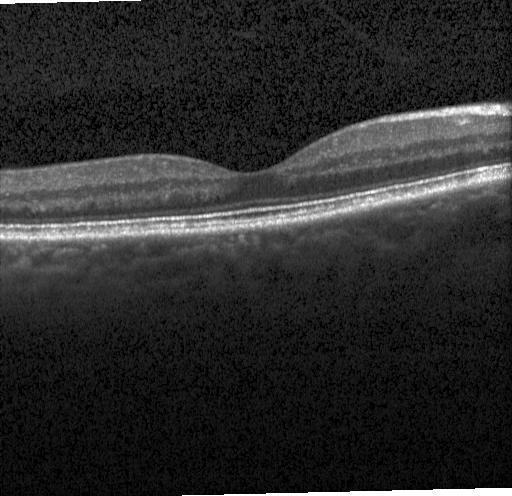

Retinal OCT cross-section · centered on the fovea · acquired on a Heidelberg Spectralis · spectral-domain OCT — The scan shows neither CNV, DME, nor drusen.